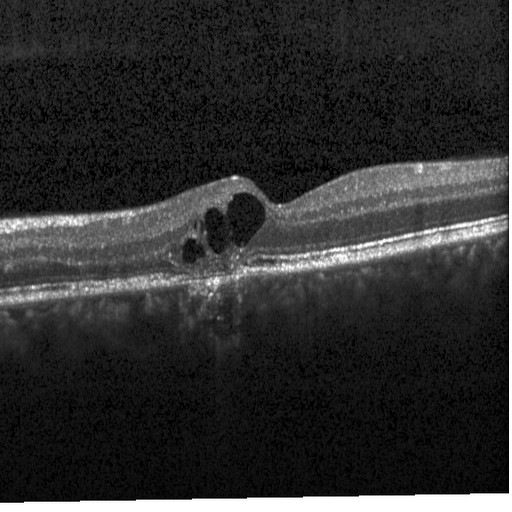

Heidelberg Spectralis; spectral-domain optical coherence tomography; macular scan; optical coherence tomography B-scan — This B-scan demonstrates DME.